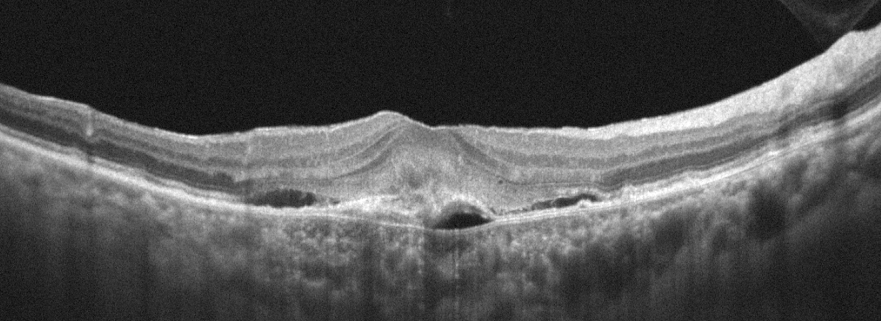
Instrument: Optovue Avanti RTVue XR · fovea-centered · retinal OCT cross-section
Impression: age-related macular degeneration.